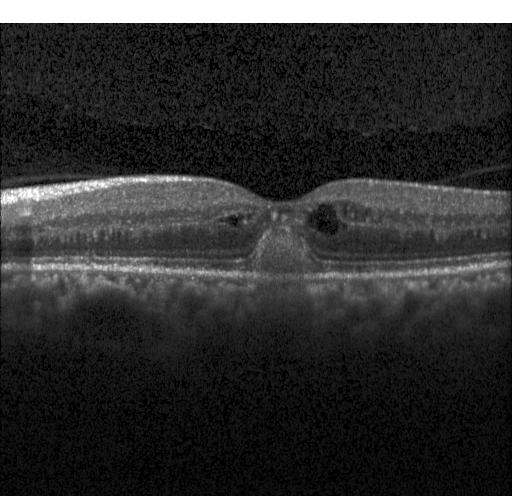 Retinal OCT cross-section · spectral-domain optical coherence tomography · acquired on a Heidelberg Spectralis · horizontal scan through the fovea. Finding: a choroidal neovascular membrane.